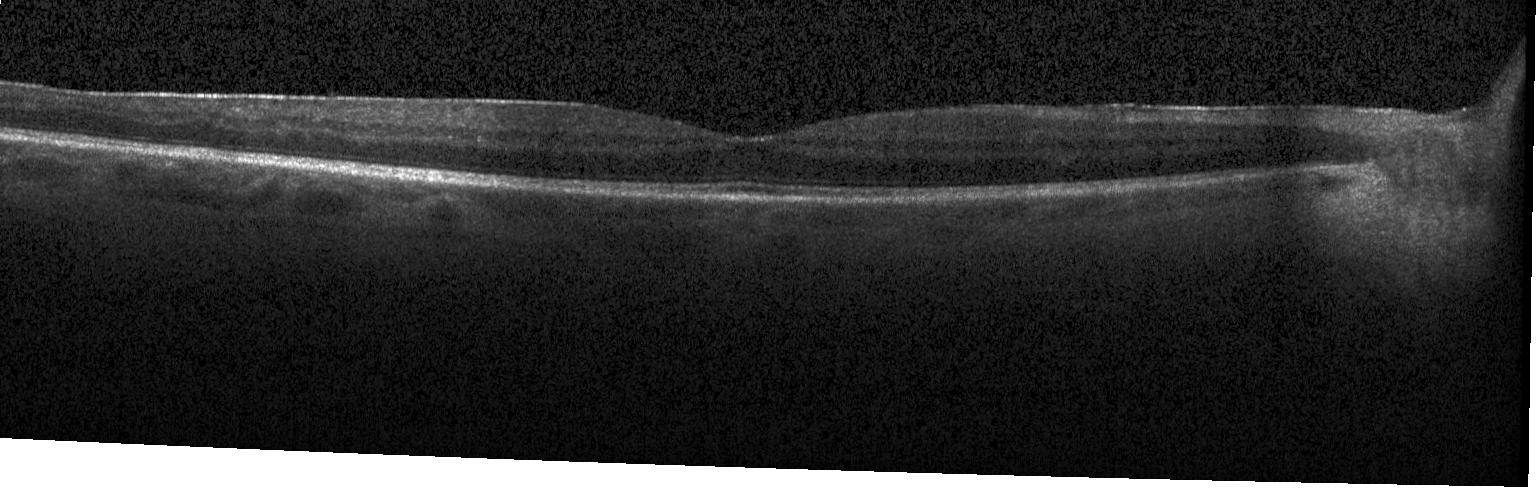 Macular scan; acquired on a Heidelberg Spectralis; OCT B-scan; spectral-domain OCT. OCT finding: no CNV, DME, or drusen.